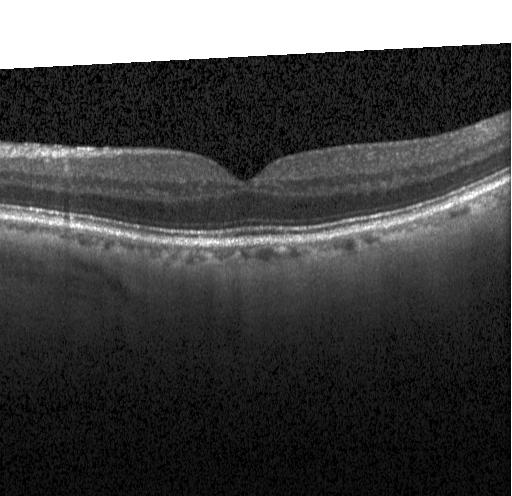
Spectral-domain OCT · Heidelberg Spectralis · centered on the fovea · optical coherence tomography B-scan. Diagnosis: no choroidal neovascularization, diabetic macular edema, or drusen.